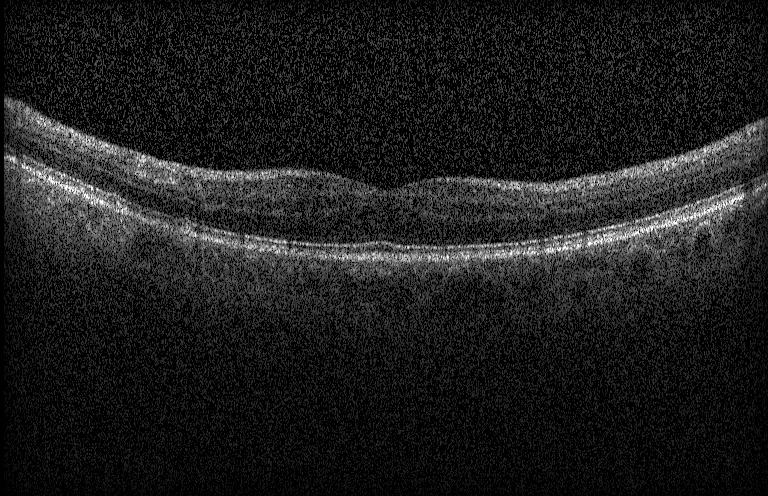

Heidelberg Spectralis OCT system; centered on the fovea; retinal OCT B-scan; spectral-domain OCT
OCT finding: no CNV, DME, or drusen.